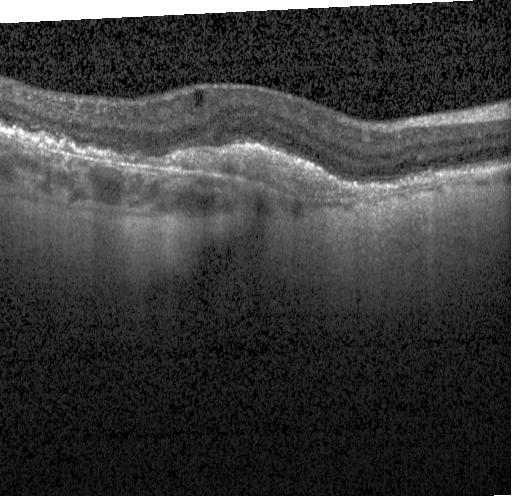
OCT line scan · spectral-domain OCT — Finding: a choroidal neovascular membrane.